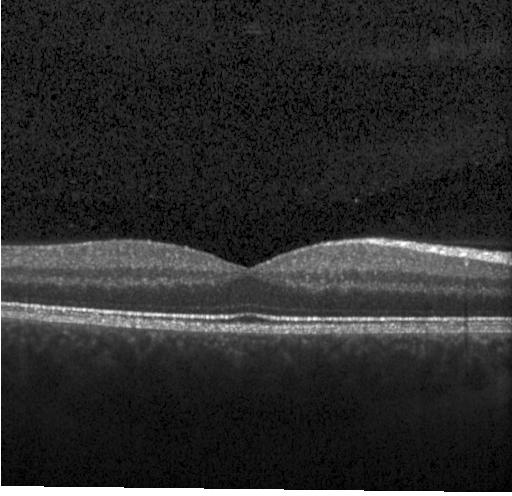 OCT line scan, horizontal scan through the fovea. Impression: no CNV, DME, or drusen.